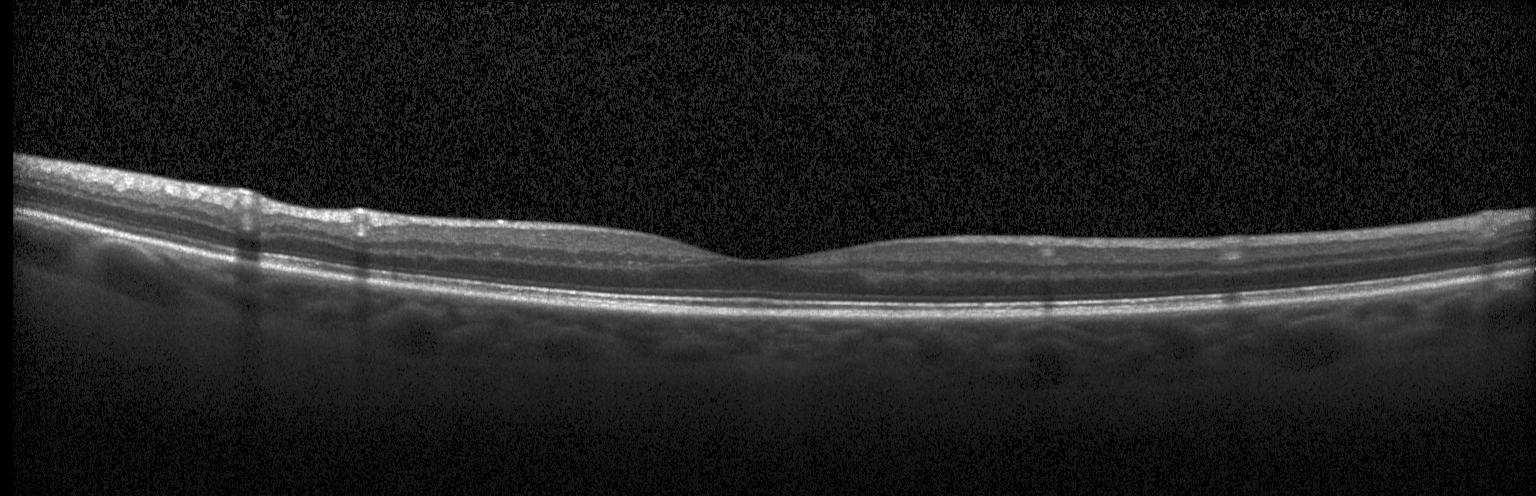

Macular OCT demonstrating neither choroidal neovascularization, diabetic macular edema, nor drusen.